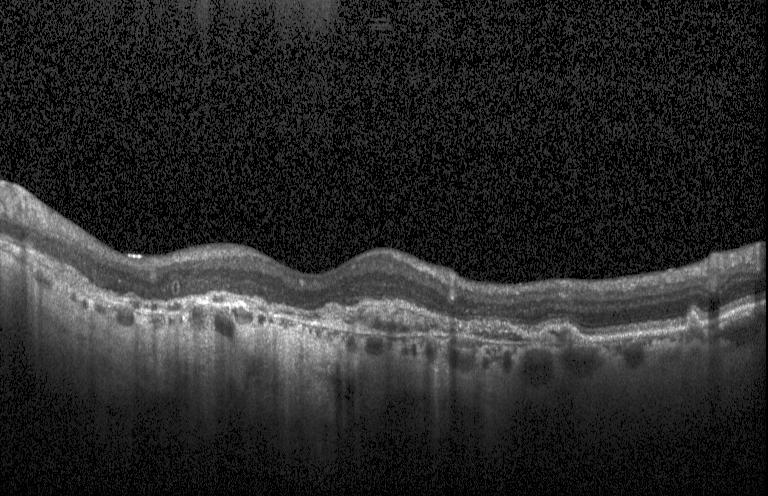

Spectral-domain optical coherence tomography, retinal OCT cross-section, Heidelberg Spectralis, fovea-centered. Assessment: choroidal neovascularization.